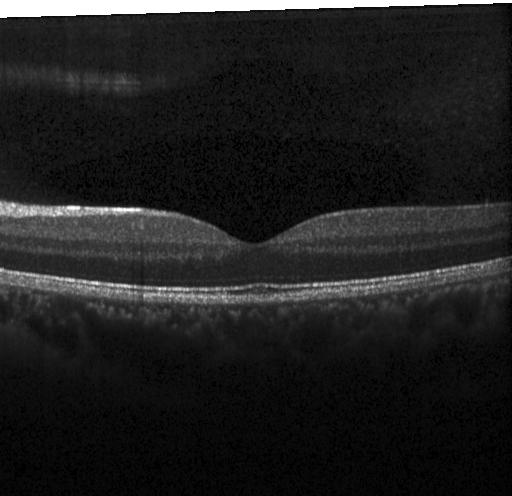

Macular OCT demonstrating no CNV, no DME, and no drusen.